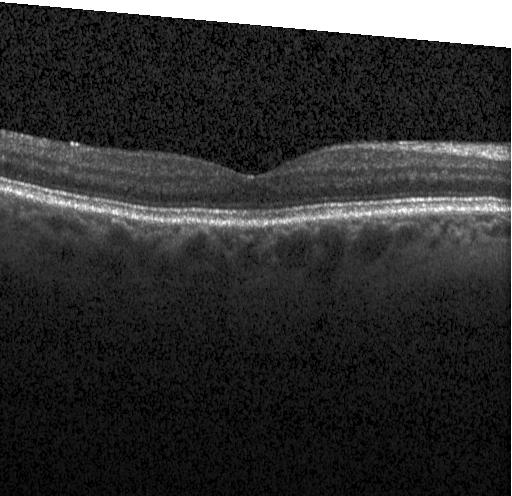
Finding: no choroidal neovascularization, diabetic macular edema, or drusen.